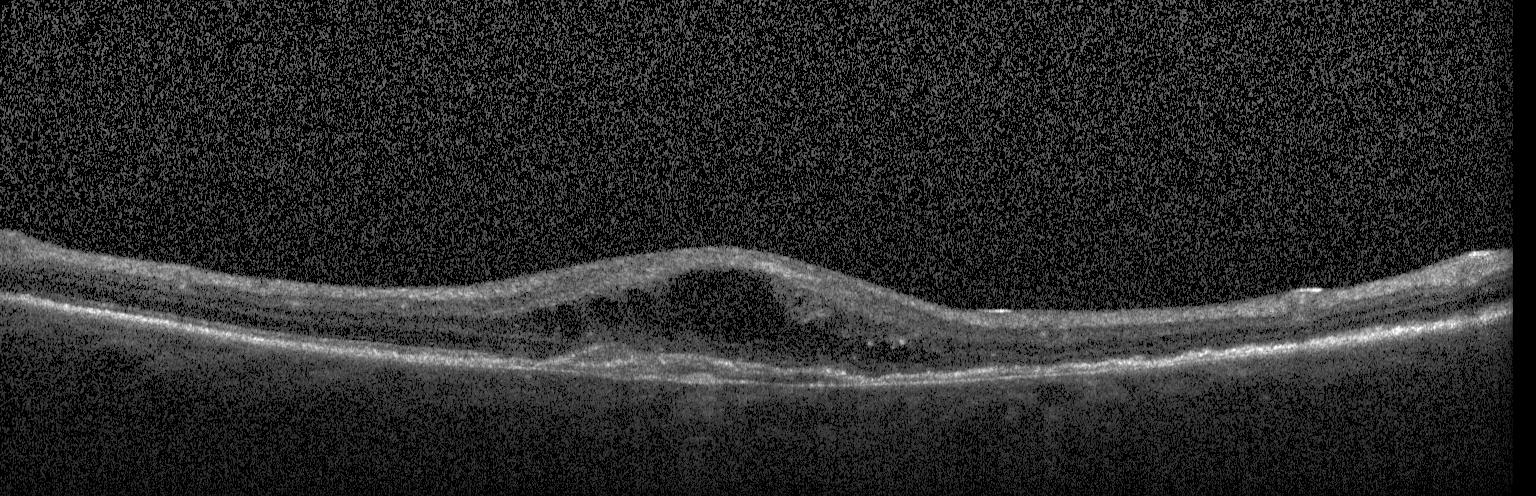

A choroidal neovascular membrane.